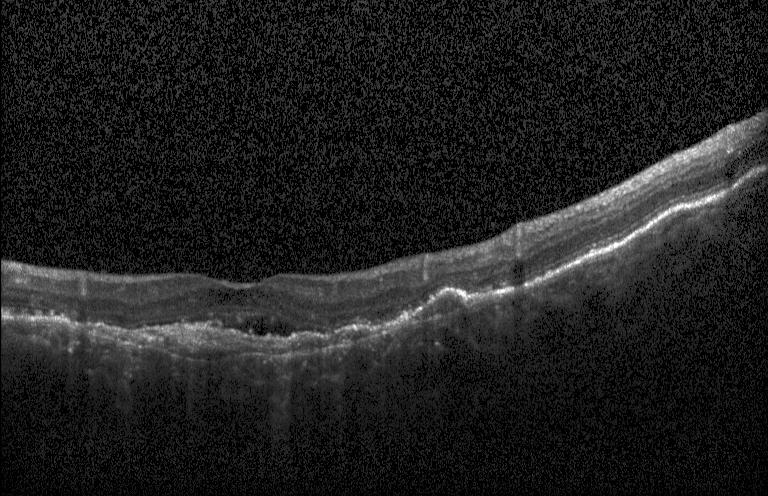
Optical coherence tomography scan.
Finding: a choroidal neovascular membrane.